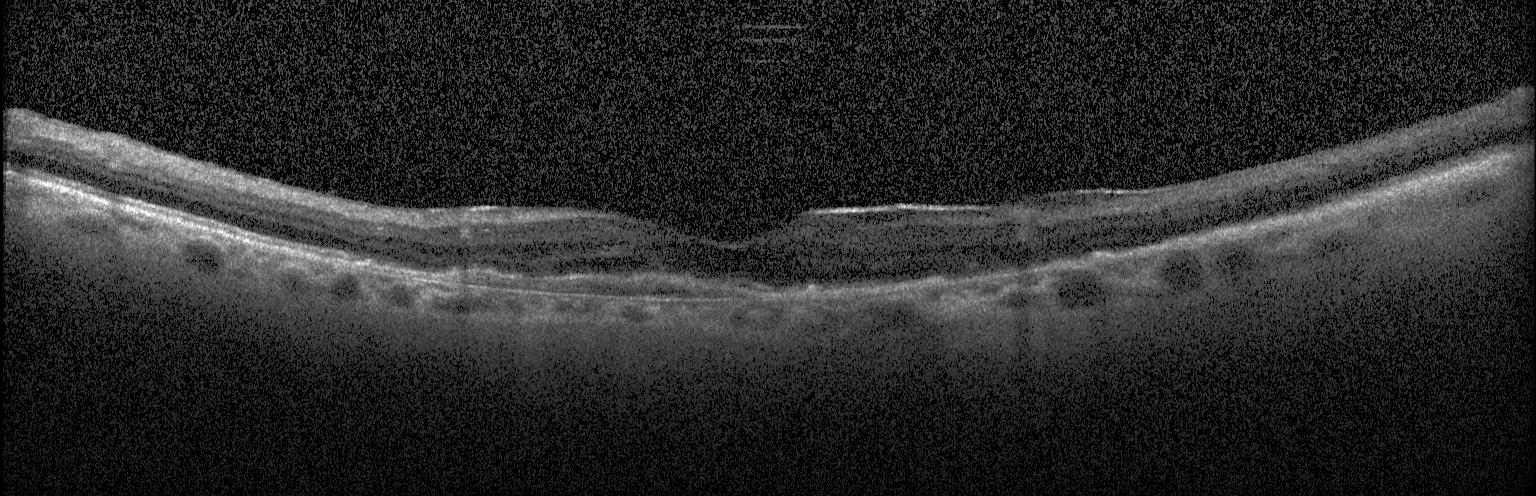

Fovea-centered. Spectral-domain optical coherence tomography. Retinal OCT cross-section — Finding: a choroidal neovascular membrane.